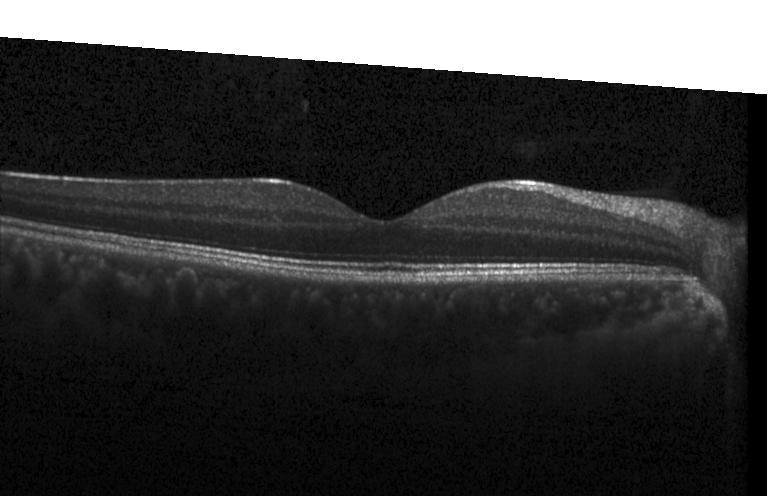 Centered on the fovea; retinal OCT B-scan; SD-OCT
This B-scan demonstrates no evidence of choroidal neovascularization, diabetic macular edema, or drusen.